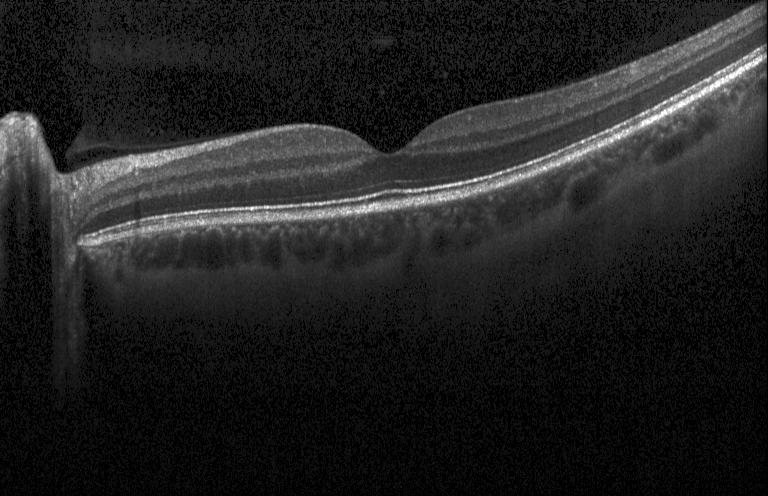 Dx: no evidence of choroidal neovascularization, diabetic macular edema, or drusen.